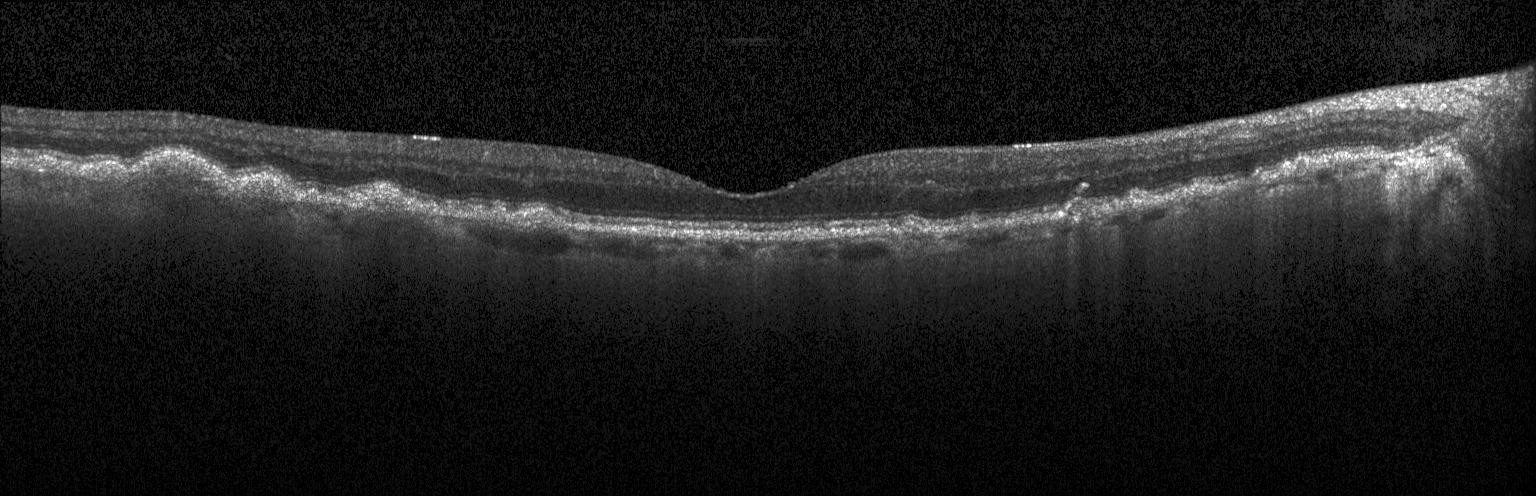 Assessment: drusen.